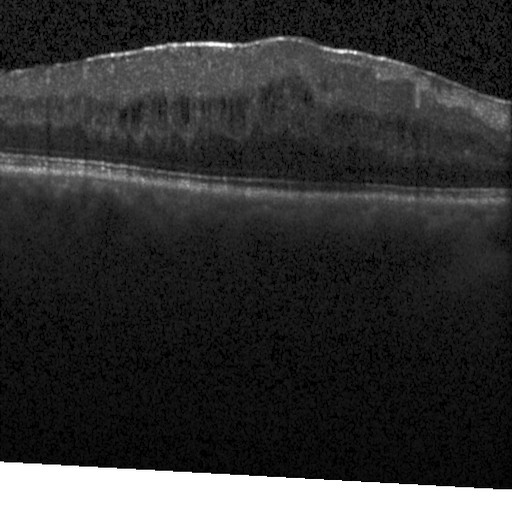
Diagnosis: diabetic macular edema (DME).